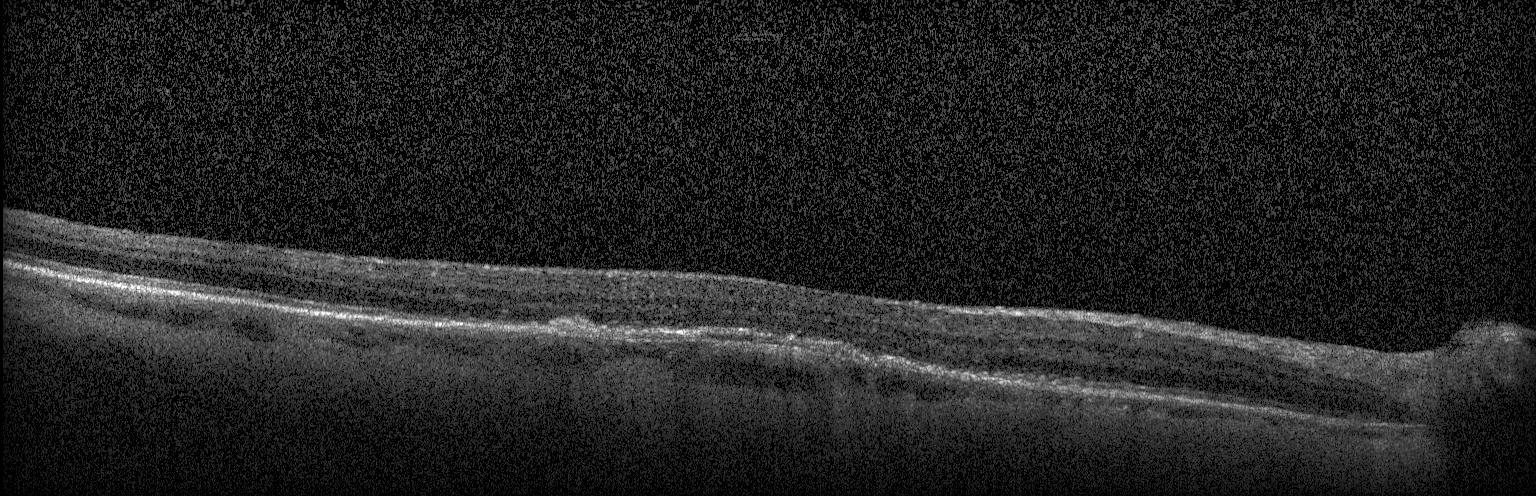 Diagnosis: a choroidal neovascular membrane.